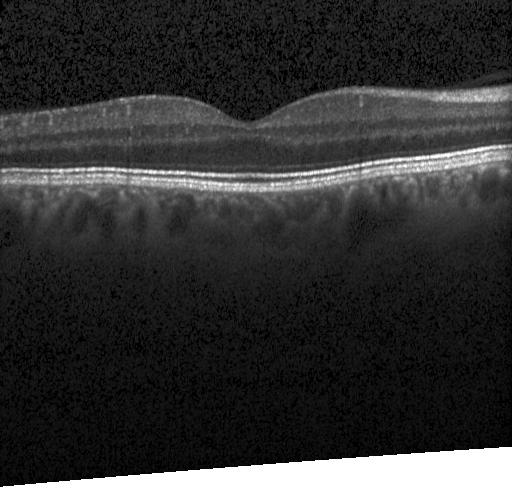 Diagnosis: no choroidal neovascularization, no diabetic macular edema, and no drusen.